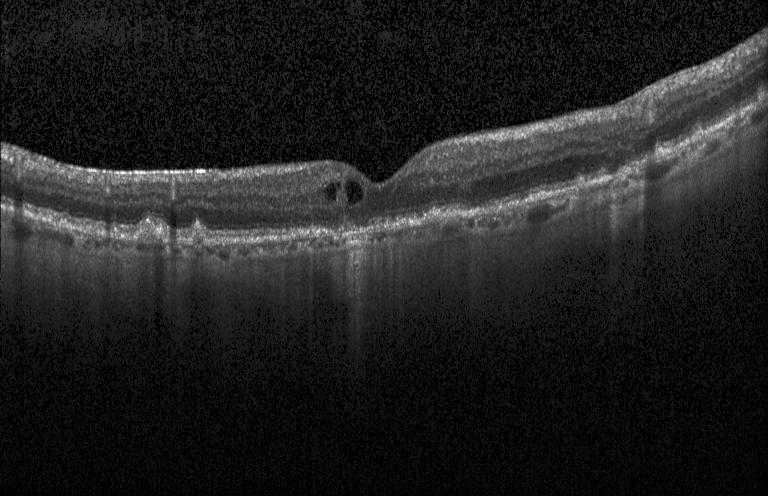

Dx: CNV.